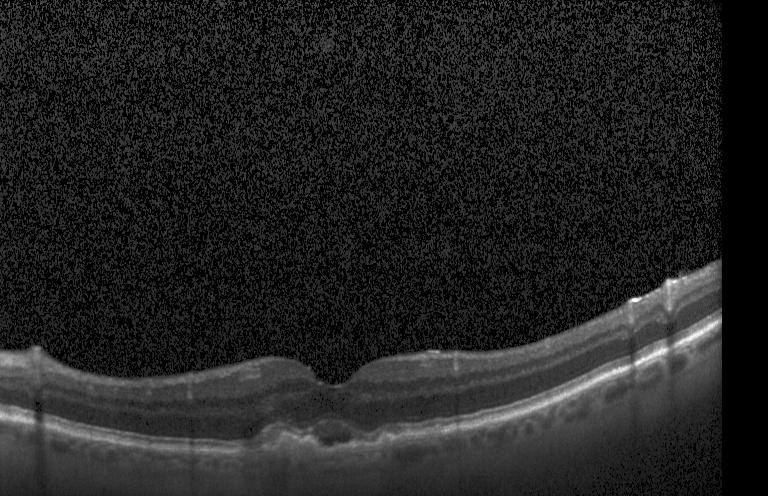
Impression: a choroidal neovascular membrane.